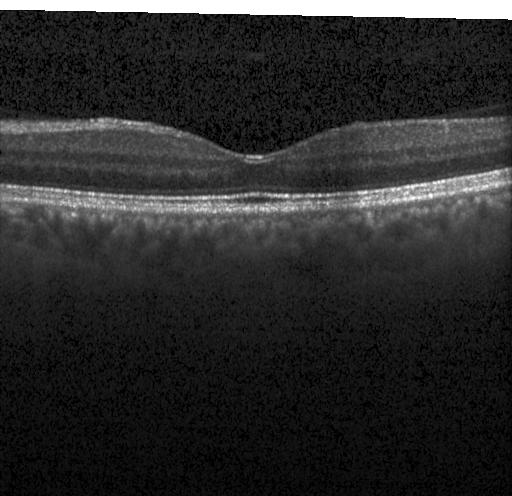
Retinal OCT B-scan. Impression: no CNV, no DME, and no drusen.